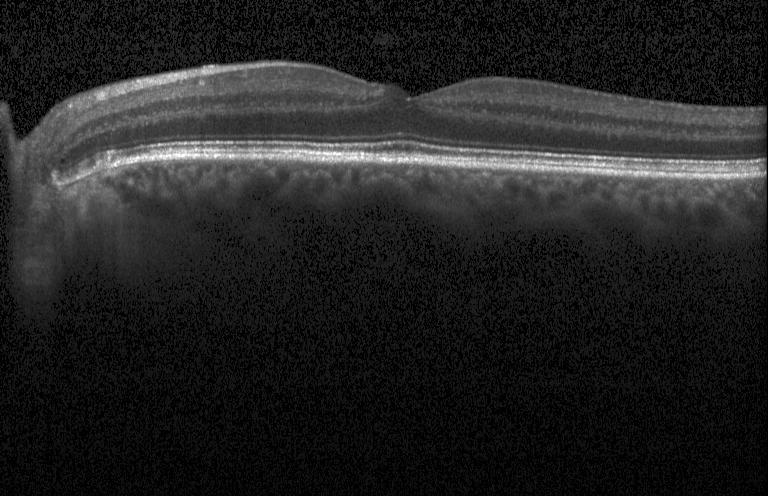 Impression: no choroidal neovascularization, diabetic macular edema, or drusen.